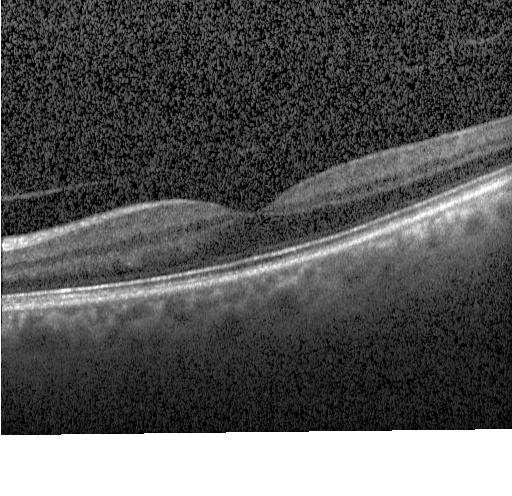
OCT finding: no choroidal neovascularization, no diabetic macular edema, and no drusen.